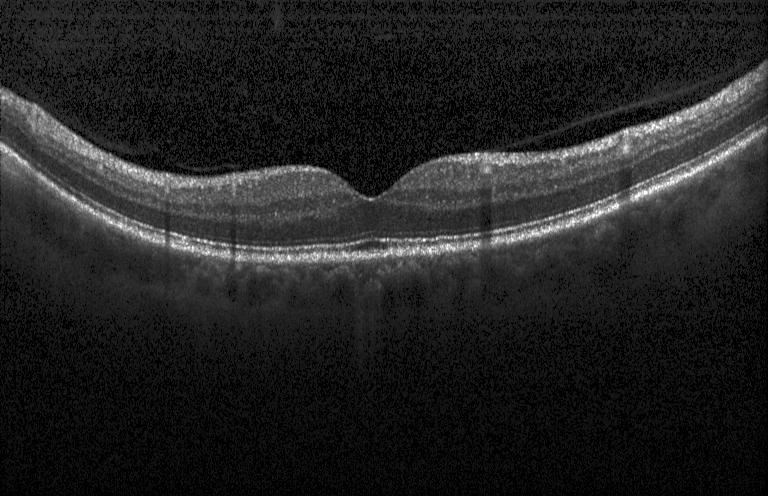
OCT scan showing no choroidal neovascularization, no diabetic macular edema, and no drusen.